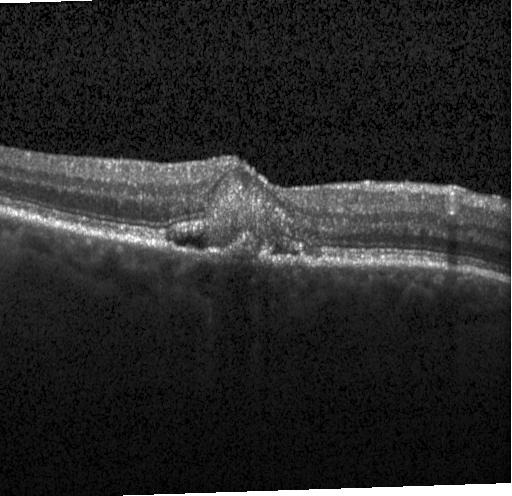

Retinal OCT B-scan.
OCT finding: a choroidal neovascular membrane.